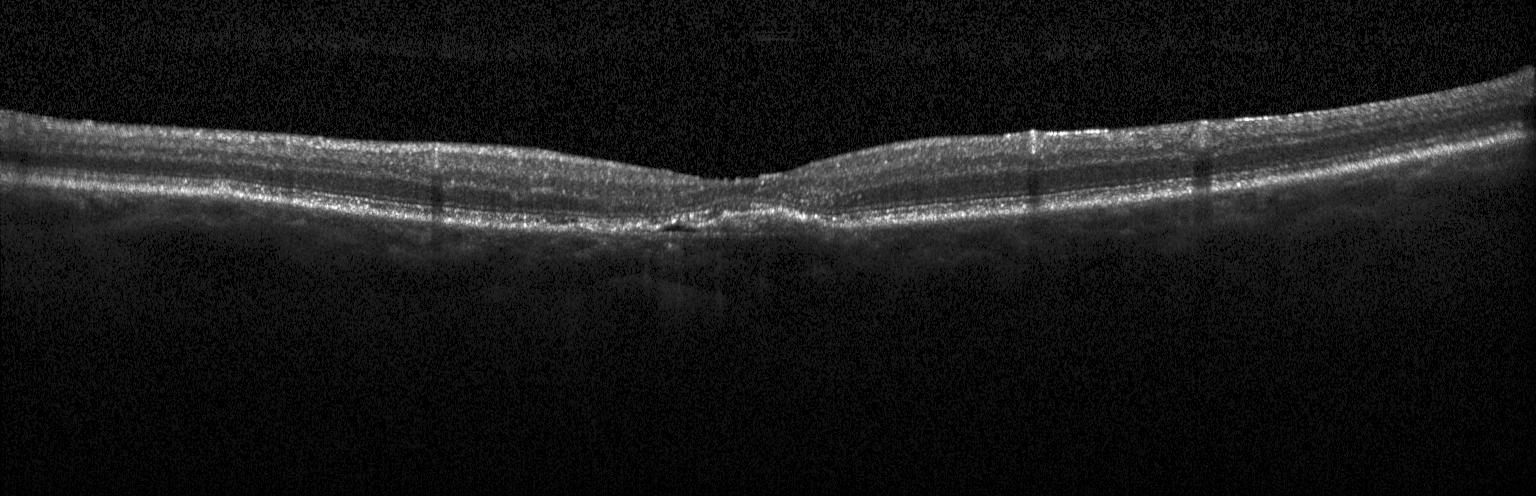 Heidelberg Spectralis; spectral-domain OCT; OCT line scan
Assessment: choroidal neovascularization (CNV).